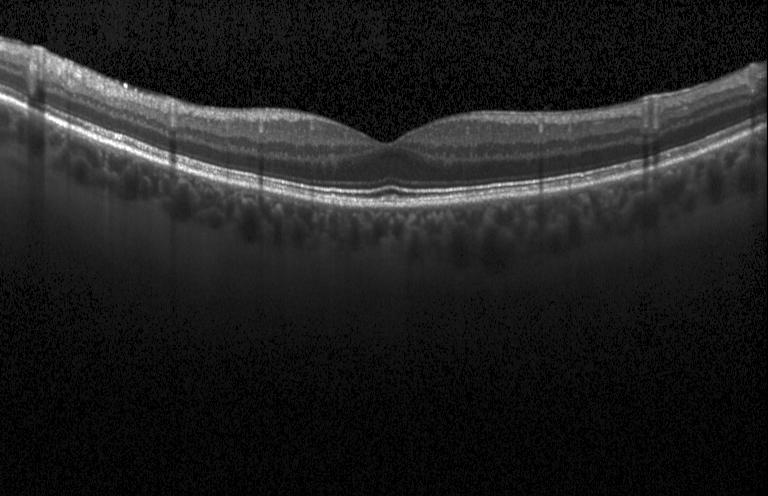
Optical coherence tomography B-scan.
Dx: no evidence of choroidal neovascularization, diabetic macular edema, or drusen.